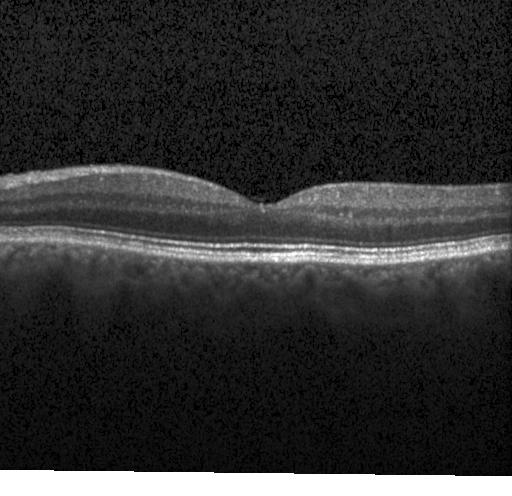 Spectral-domain optical coherence tomography; Heidelberg Spectralis OCT system; retinal OCT B-scan. The scan shows neither choroidal neovascularization, diabetic macular edema, nor drusen.